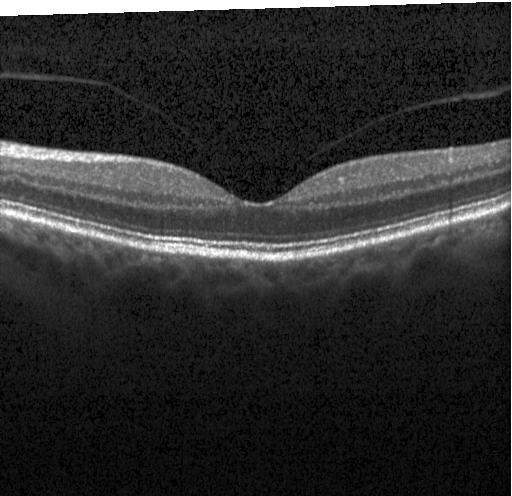

OCT line scan, centered on the fovea. Dx: neither choroidal neovascularization, diabetic macular edema, nor drusen.